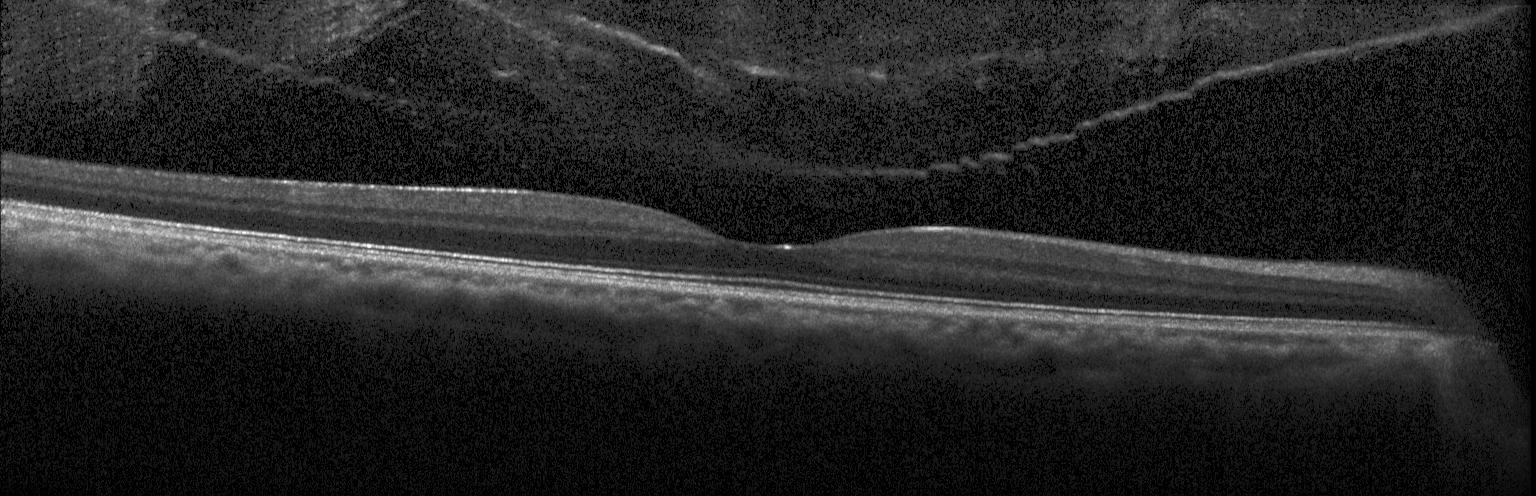
Macular OCT demonstrating no evidence of CNV, DME, or drusen.